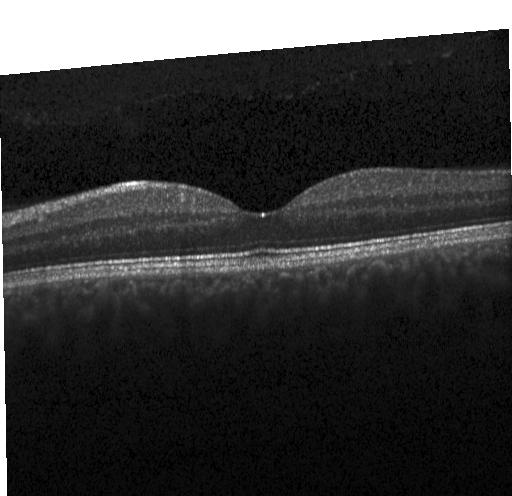 Optical coherence tomography B-scan
Finding: no CNV, no DME, and no drusen.